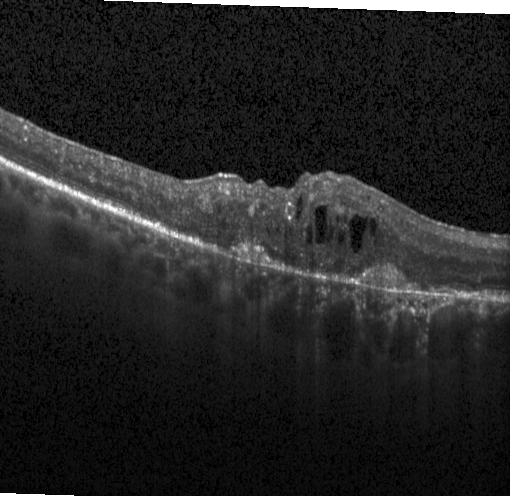

OCT line scan; horizontal scan through the fovea.
The scan shows choroidal neovascularization (CNV).